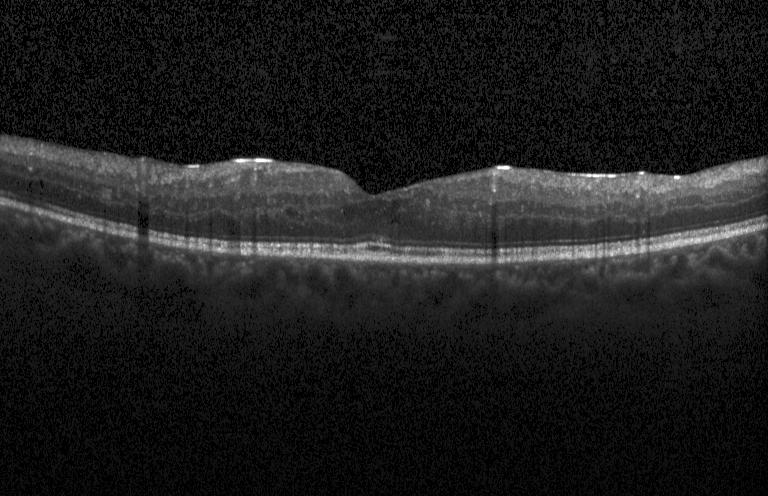
OCT line scan
Impression: diabetic macular edema (DME).